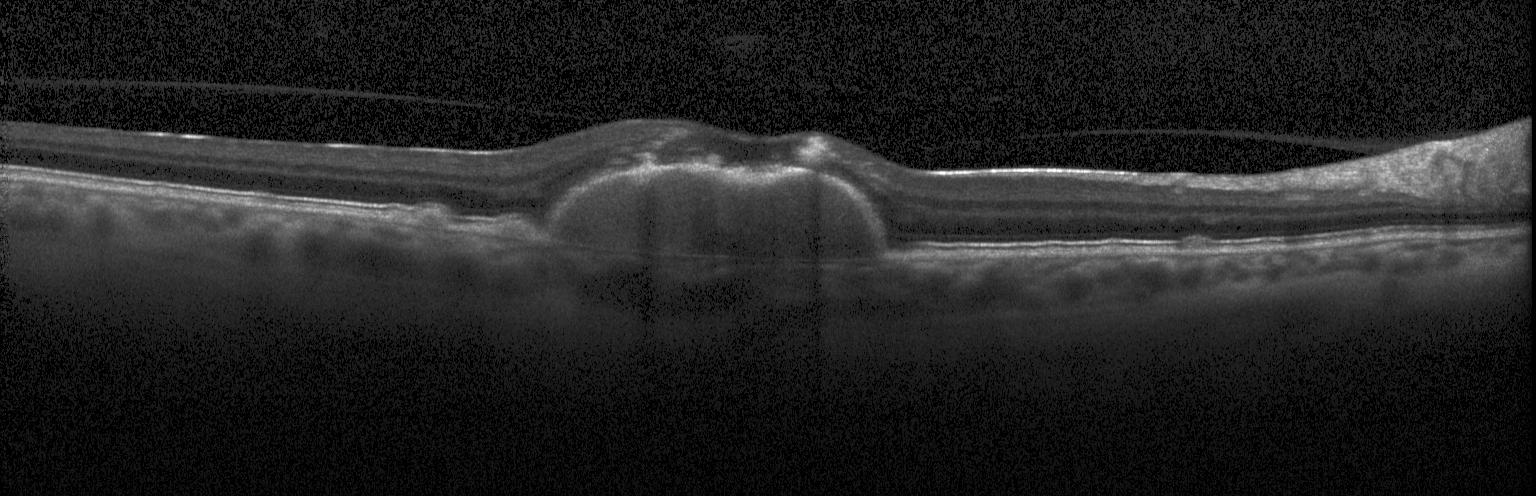 Macular OCT: choroidal neovascularization.